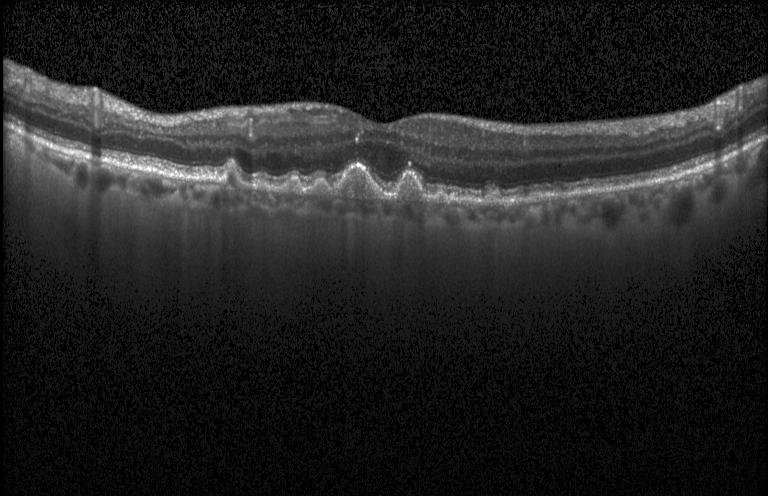

SD-OCT. OCT B-scan.
Finding: multiple drusen.